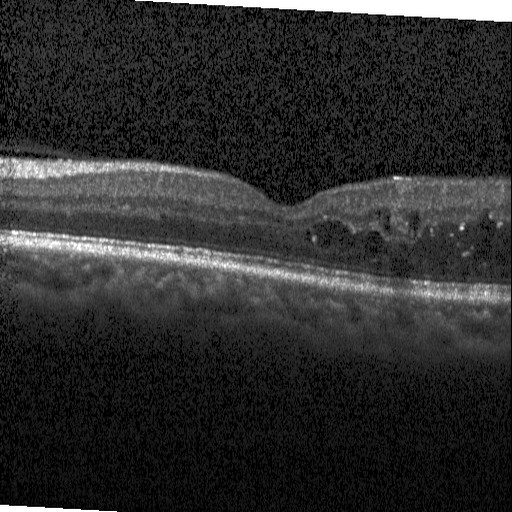 Spectral-domain optical coherence tomography · OCT B-scan · instrument: Heidelberg Spectralis.
Macular OCT: DME.